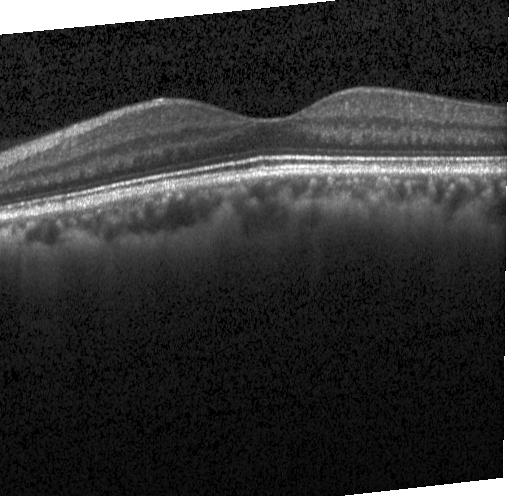
Optical coherence tomography scan. Heidelberg Spectralis. Assessment: no CNV, no DME, and no drusen.